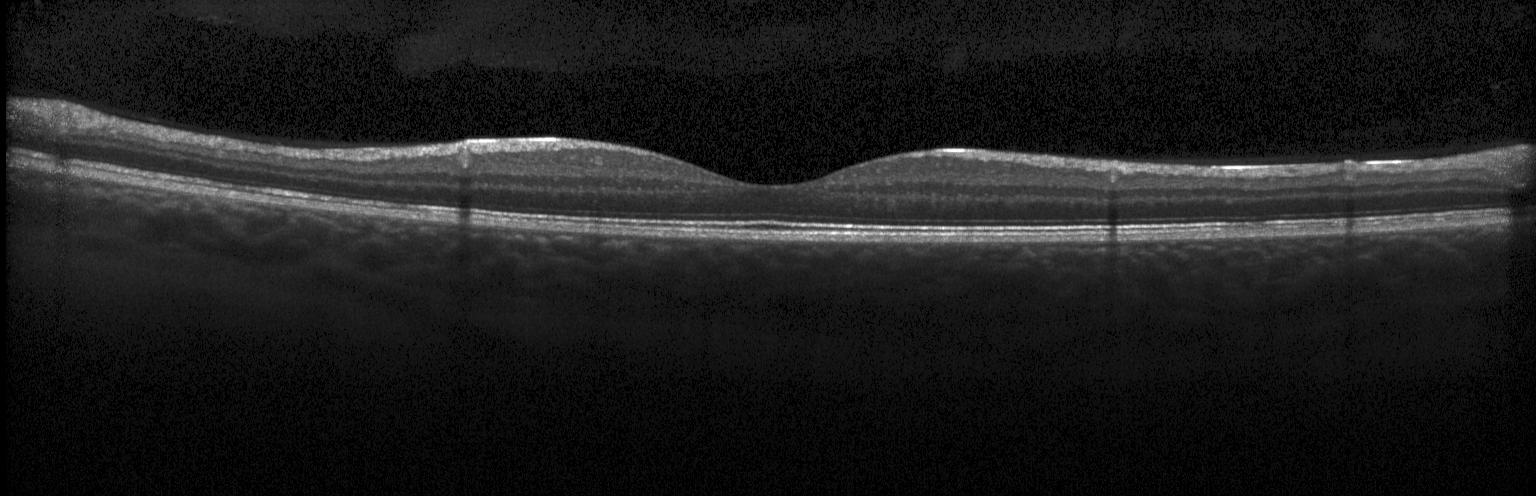
Spectral-domain OCT B-scan: no choroidal neovascularization, no diabetic macular edema, and no drusen.